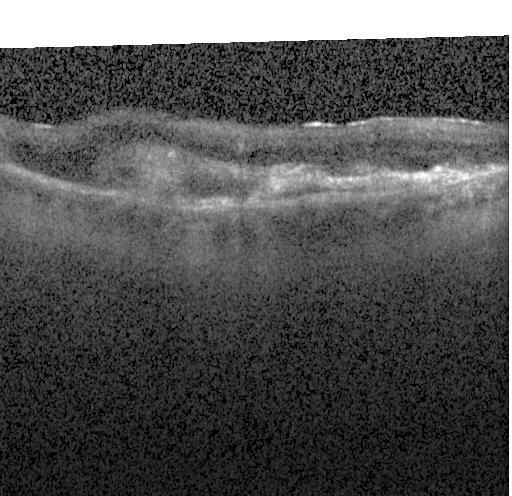 Macular scan, retinal OCT cross-section.
Assessment: a choroidal neovascular membrane.